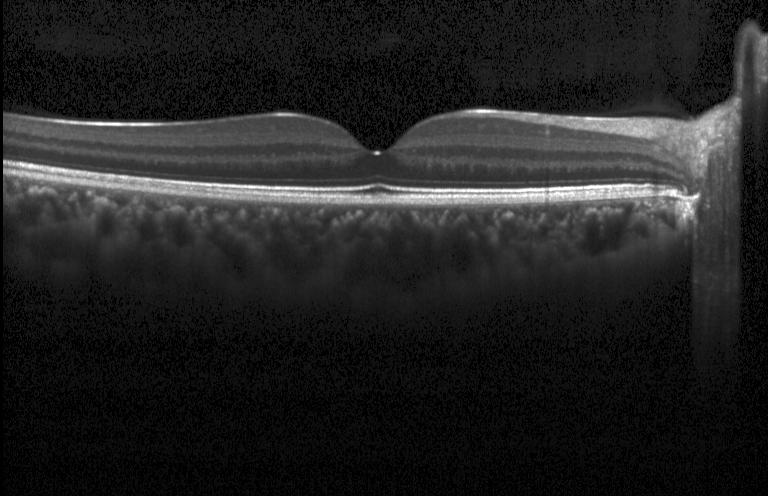 Retinal OCT cross-section showing neither CNV, DME, nor drusen.